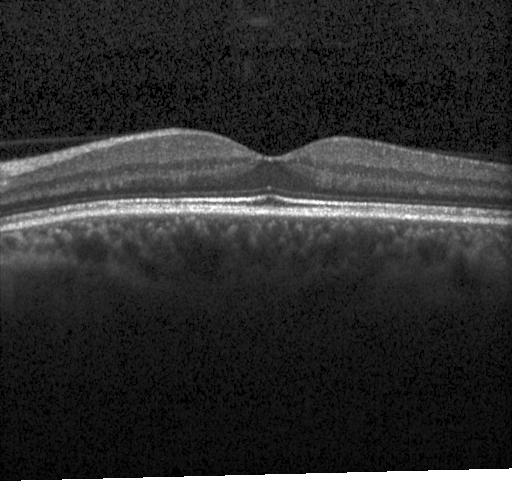 Impression: no CNV, no DME, and no drusen.